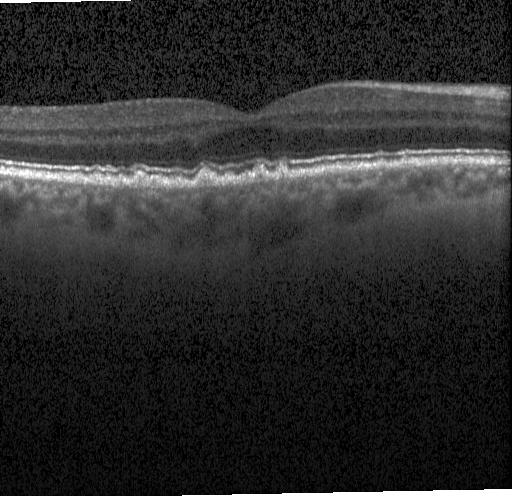

Fovea-centered · OCT B-scan
OCT finding: drusen.